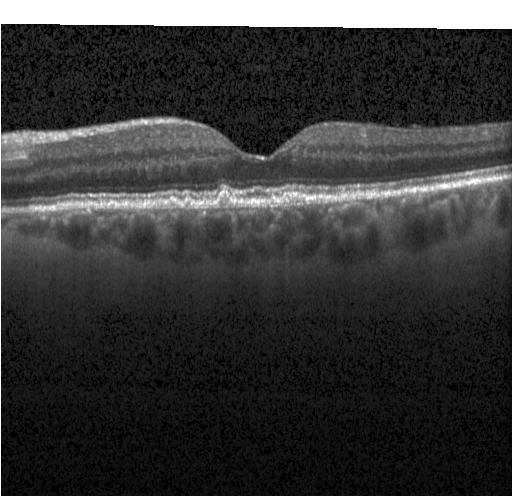
Instrument: Heidelberg Spectralis; optical coherence tomography B-scan; macular scan
The scan shows multiple drusen.